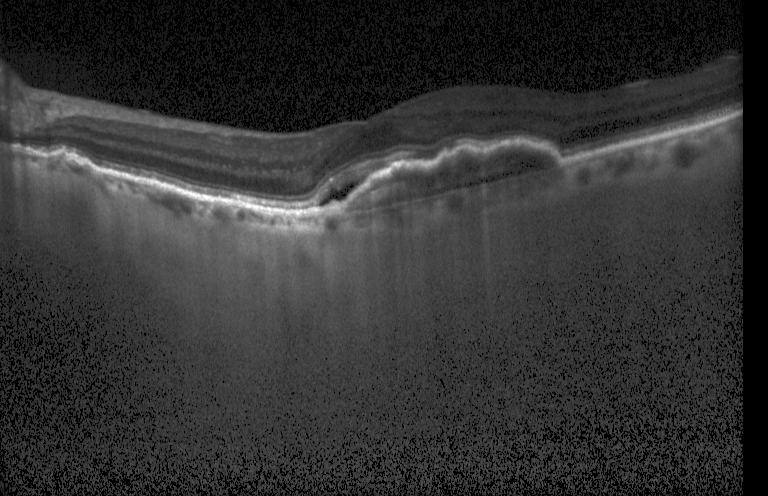
OCT line scan.
Finding: CNV.